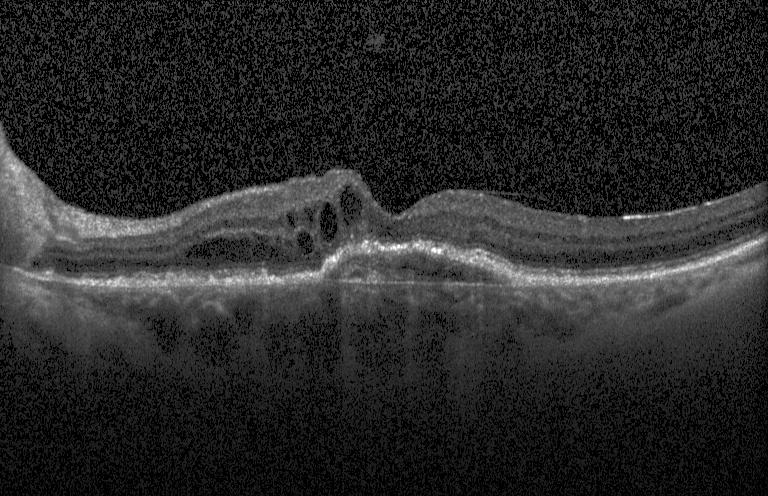 SD-OCT · Heidelberg Spectralis OCT system · optical coherence tomography scan · horizontal scan through the fovea. Impression: CNV.